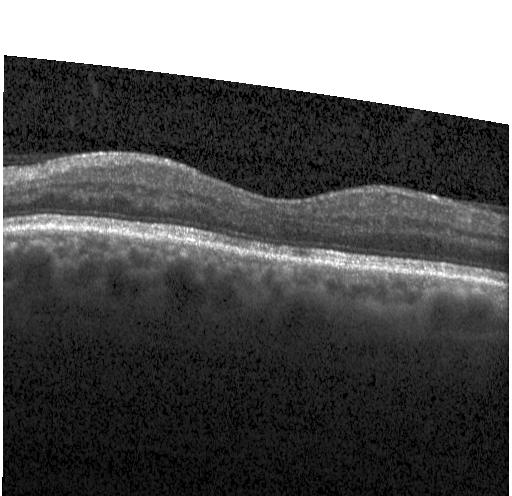

Retinal OCT cross-section.
Finding: no evidence of choroidal neovascularization, diabetic macular edema, or drusen.